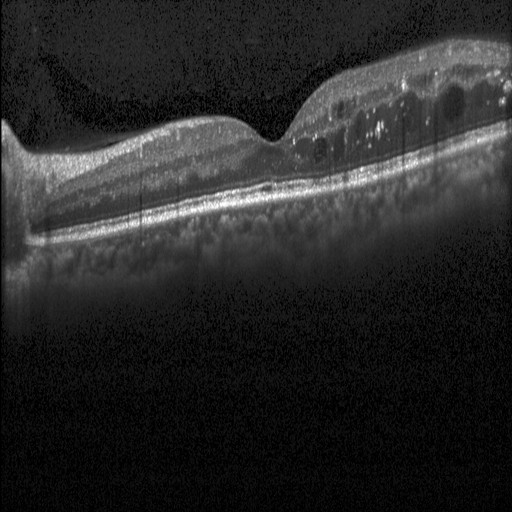

Impression: diabetic macular edema (DME).